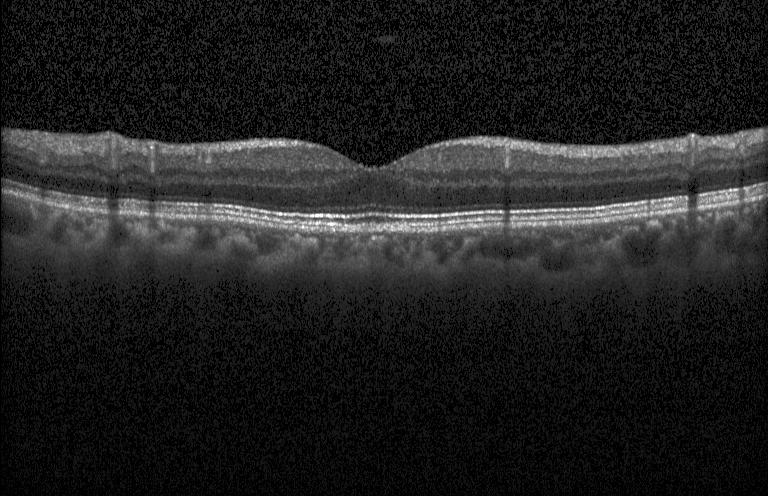 Macular OCT demonstrating no evidence of choroidal neovascularization, diabetic macular edema, or drusen.